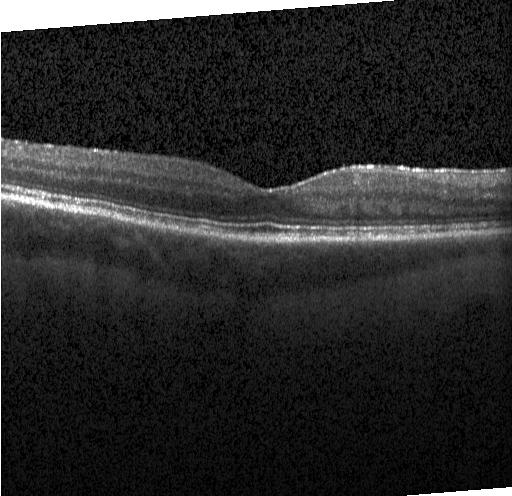 OCT scan showing no choroidal neovascularization, diabetic macular edema, or drusen.